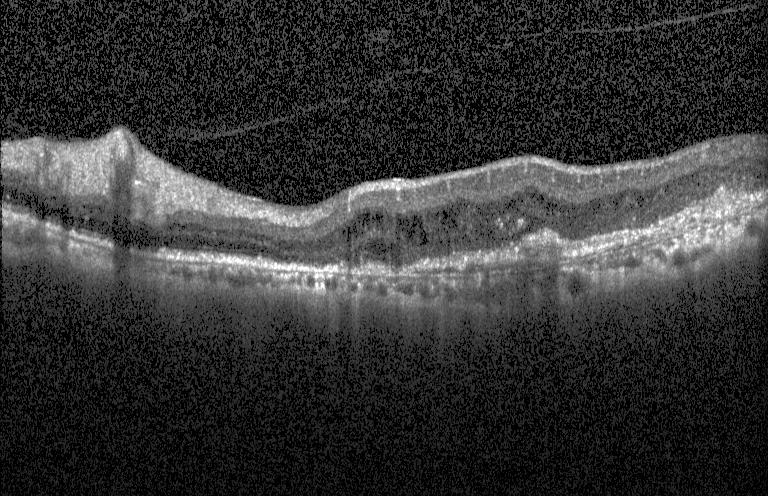 Spectral-domain OCT; retinal OCT B-scan; Heidelberg Spectralis OCT system; macular scan — Assessment: choroidal neovascularization.